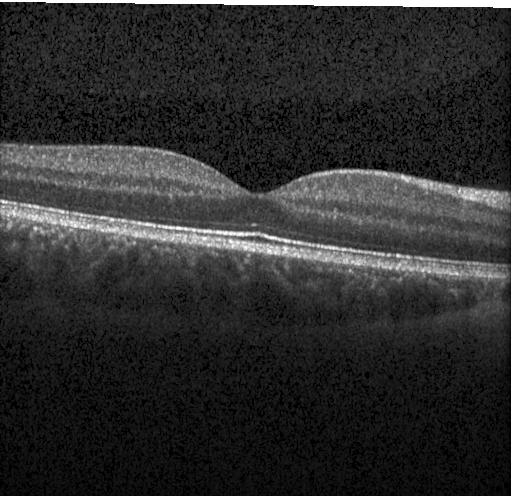

Impression: no CNV, no DME, and no drusen.